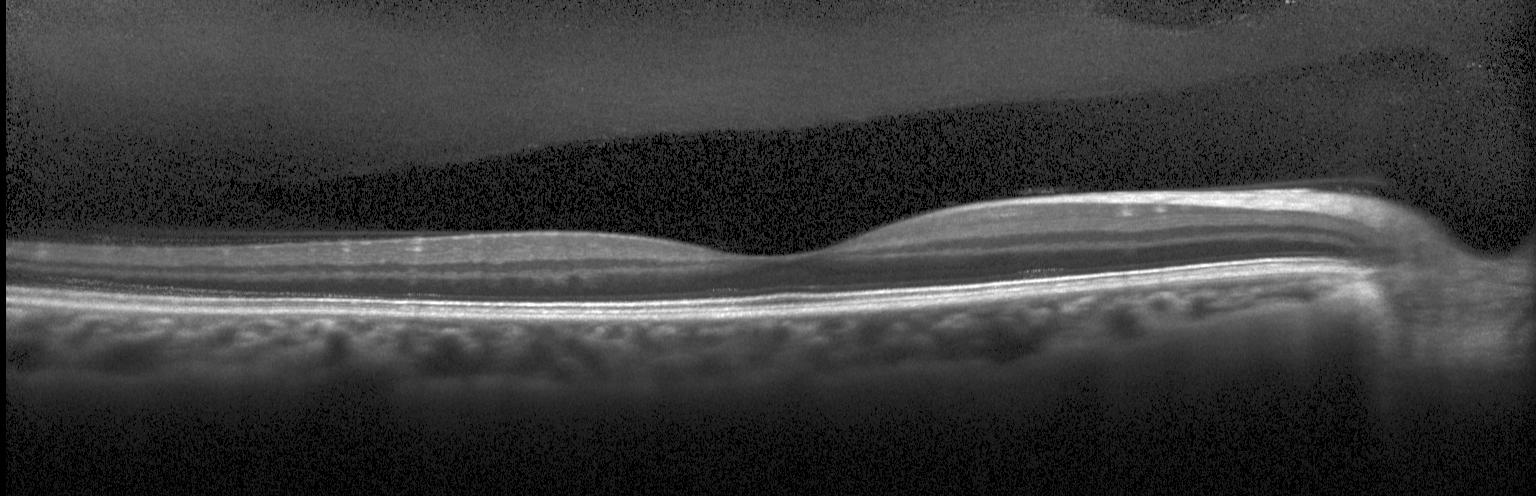

Retinal OCT B-scan
Finding: no choroidal neovascularization, diabetic macular edema, or drusen.